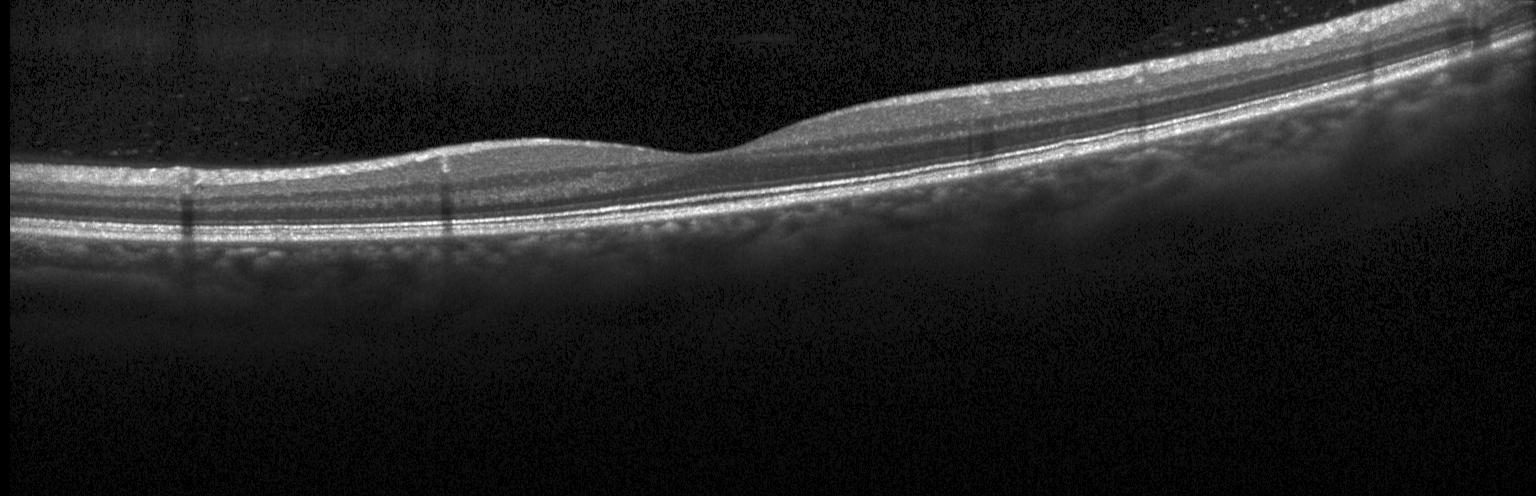 Retinal OCT cross-section showing neither choroidal neovascularization, diabetic macular edema, nor drusen.